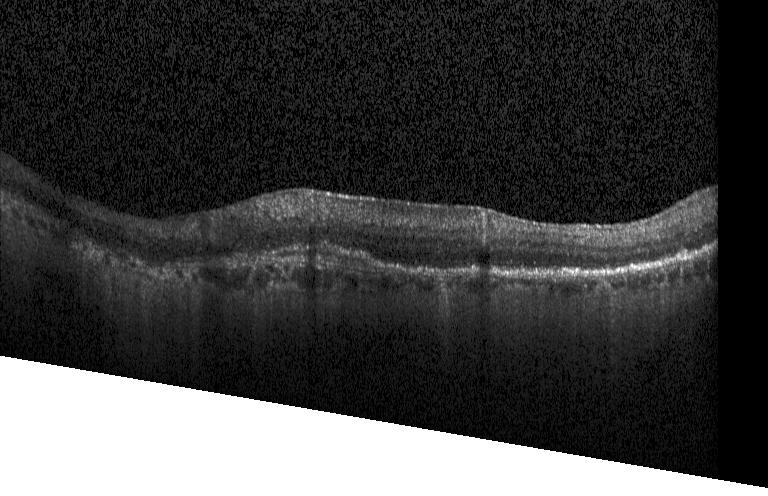

OCT line scan
This B-scan demonstrates choroidal neovascularization.